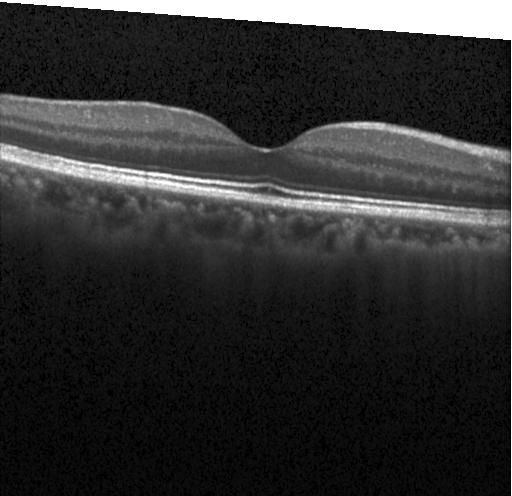 Impression: neither choroidal neovascularization, diabetic macular edema, nor drusen.